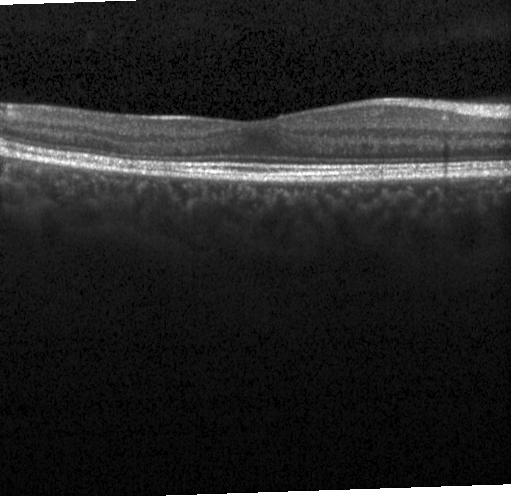
OCT line scan
This B-scan demonstrates no choroidal neovascularization, no diabetic macular edema, and no drusen.